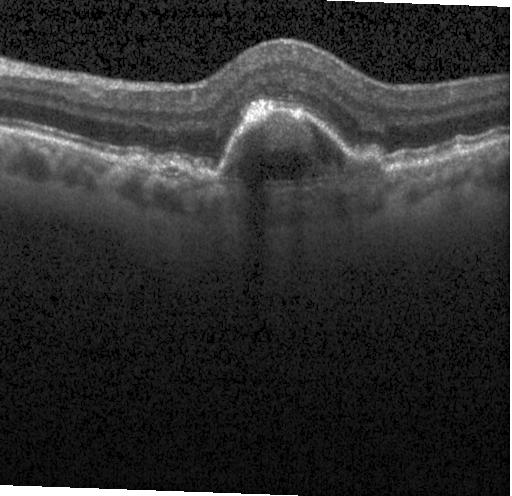
Spectral-domain OCT. Acquired on a Heidelberg Spectralis. Fovea-centered. Optical coherence tomography scan — Impression: drusen.